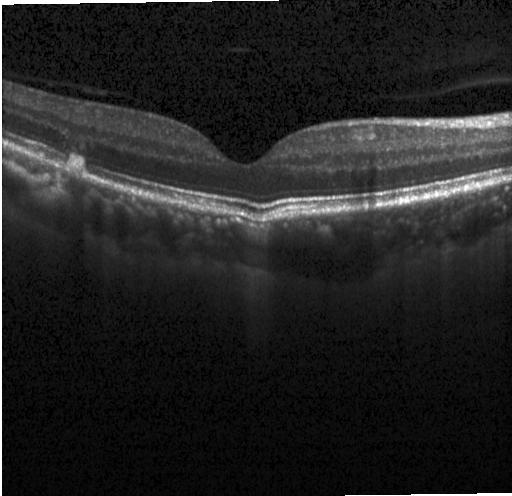
Macular scan; OCT B-scan.
Impression: sub-RPE drusenoid deposits.